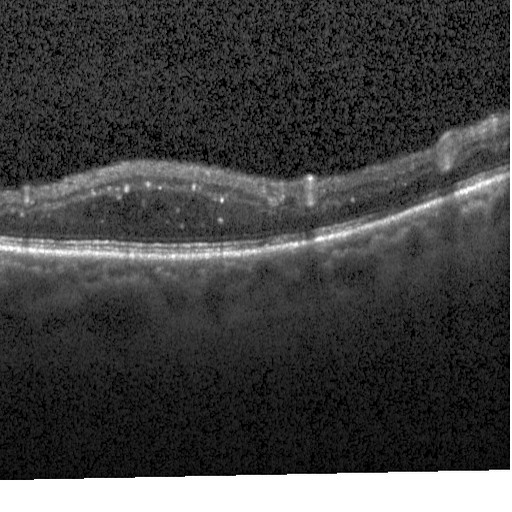
Spectral-domain OCT B-scan: diabetic macular edema (DME).